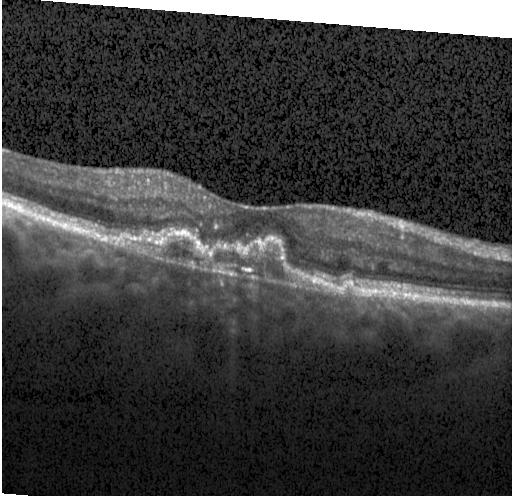
Spectral-domain OCT, OCT B-scan, horizontal scan through the fovea, Heidelberg Spectralis. Choroidal neovascularization (CNV).